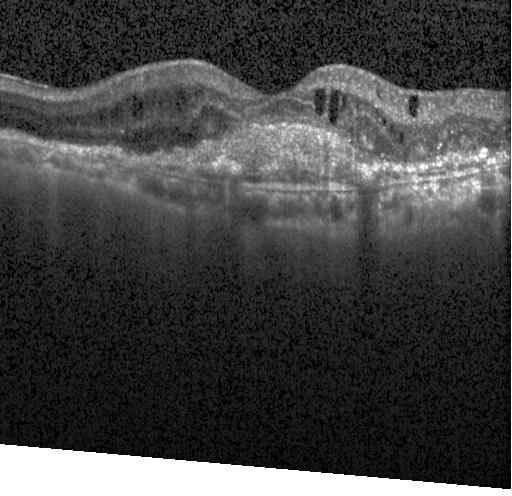
SD-OCT, macular scan, acquired on a Heidelberg Spectralis, OCT B-scan
Assessment: a choroidal neovascular membrane.